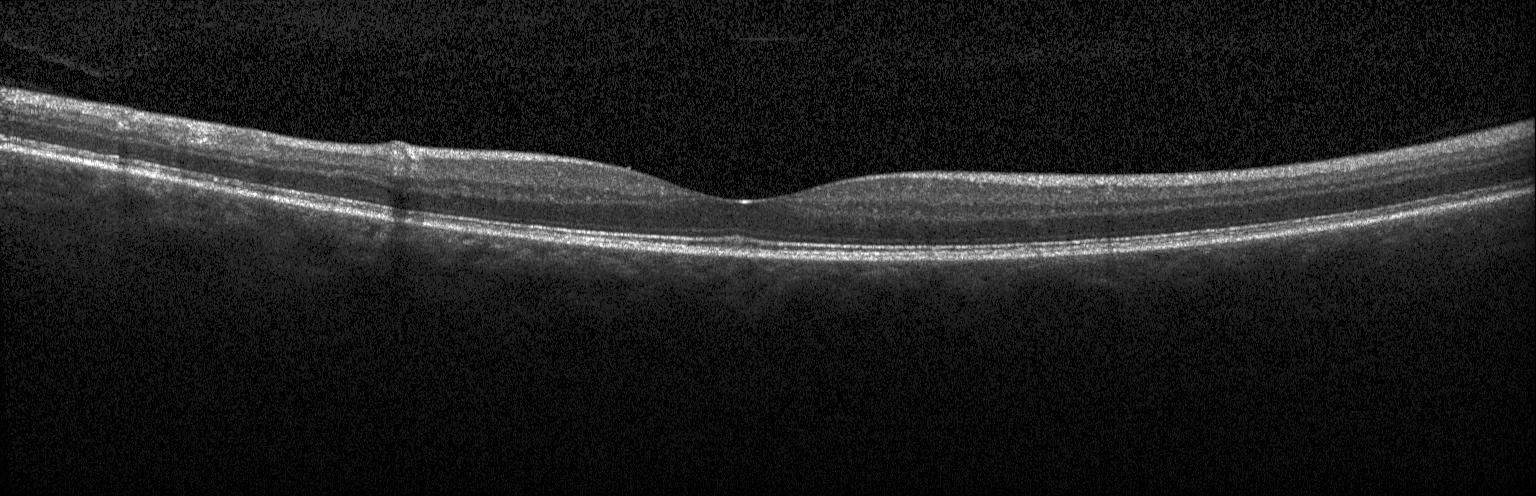

Impression: no evidence of choroidal neovascularization, diabetic macular edema, or drusen.